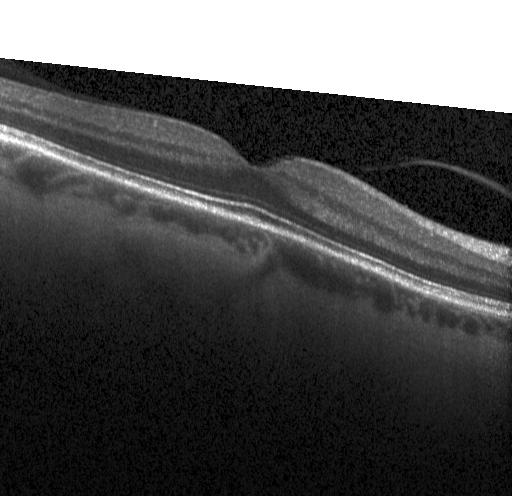

Impression: no evidence of choroidal neovascularization, diabetic macular edema, or drusen.